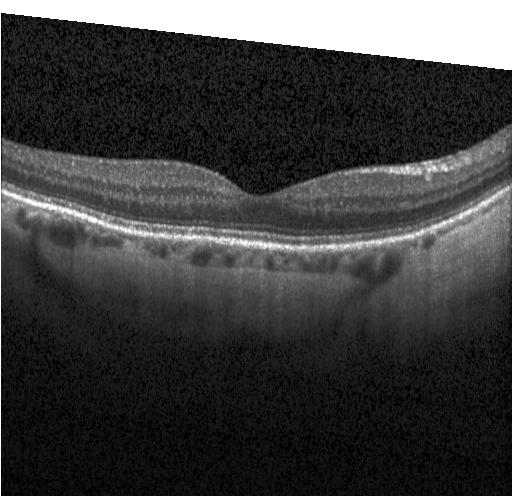

Retinal OCT cross-section showing no evidence of CNV, DME, or drusen.